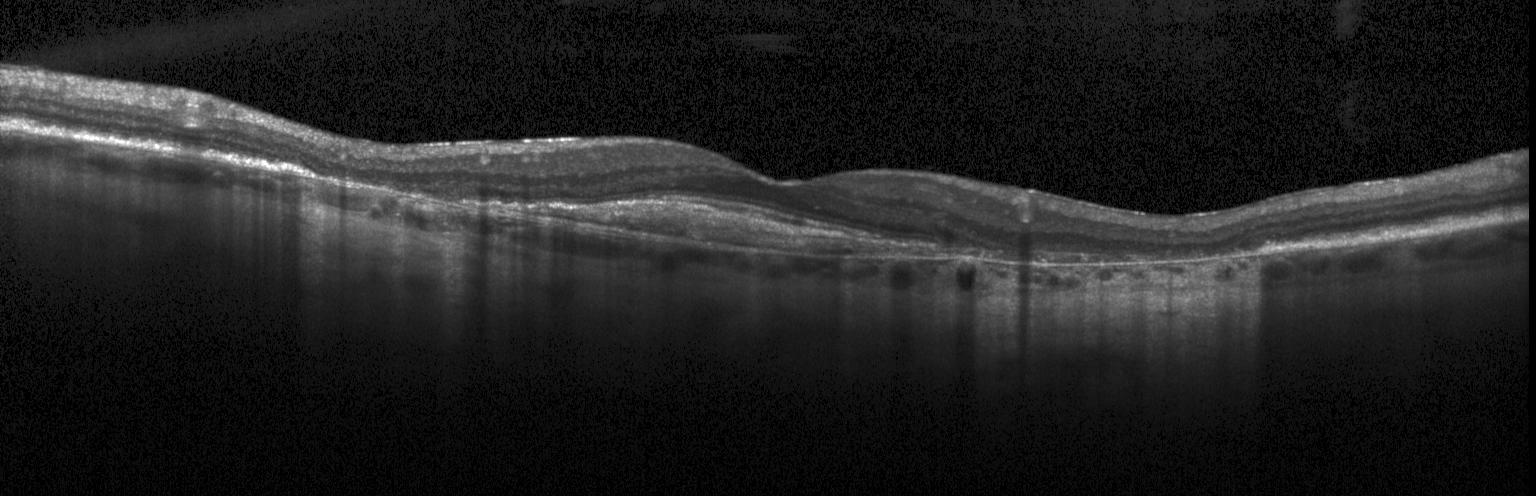
A choroidal neovascular membrane.